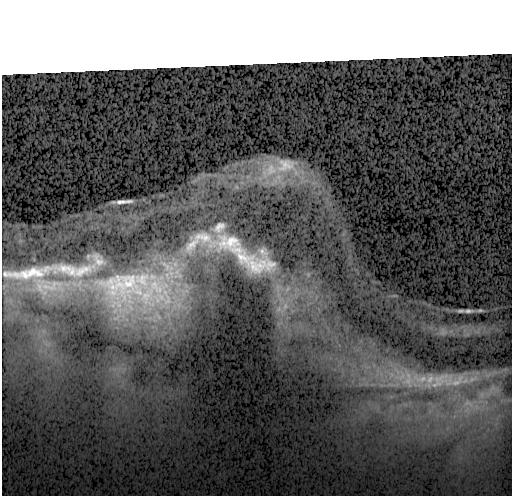
Retinal OCT B-scan.
Diagnosis: a choroidal neovascular membrane.